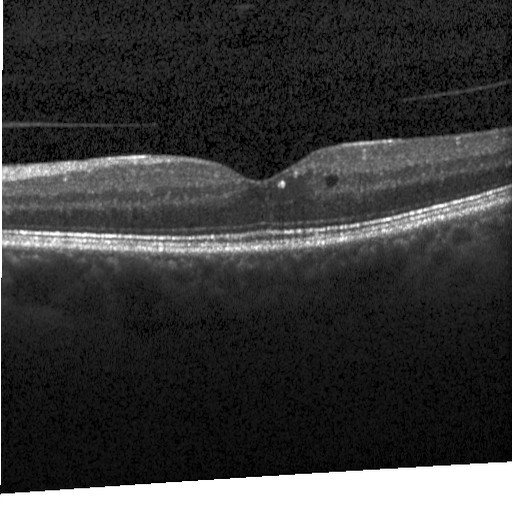
Spectral-domain optical coherence tomography · optical coherence tomography B-scan · Heidelberg Spectralis.
Impression: DME.